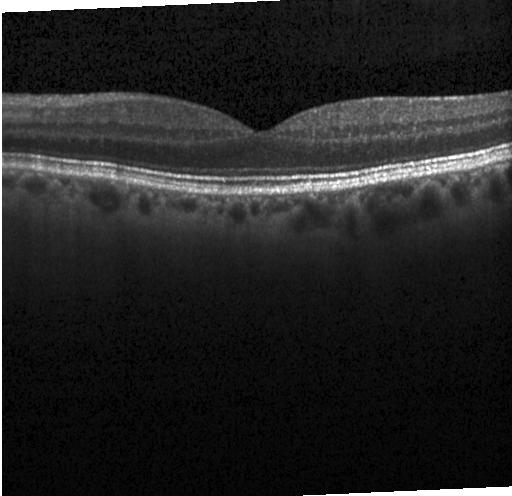 Instrument: Heidelberg Spectralis, retinal OCT B-scan. Diagnosis: no choroidal neovascularization, no diabetic macular edema, and no drusen.